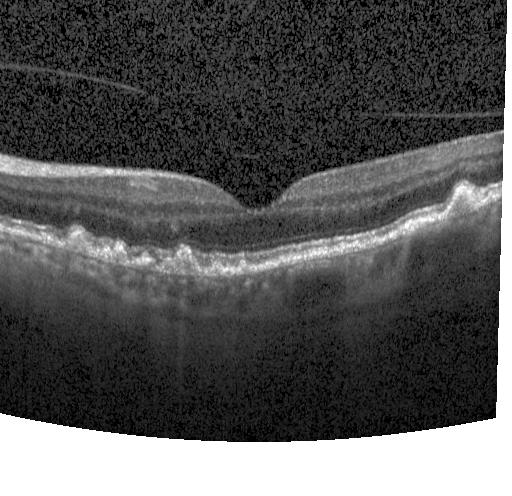 Diagnosis: drusen.